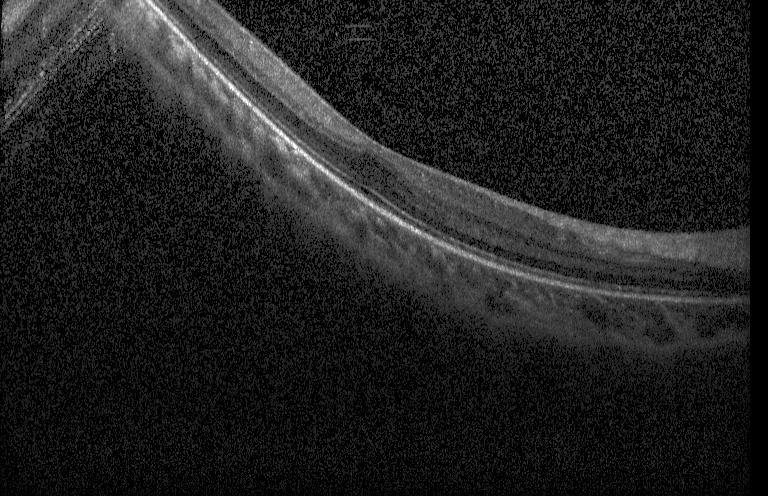

Impression: no evidence of choroidal neovascularization, diabetic macular edema, or drusen.